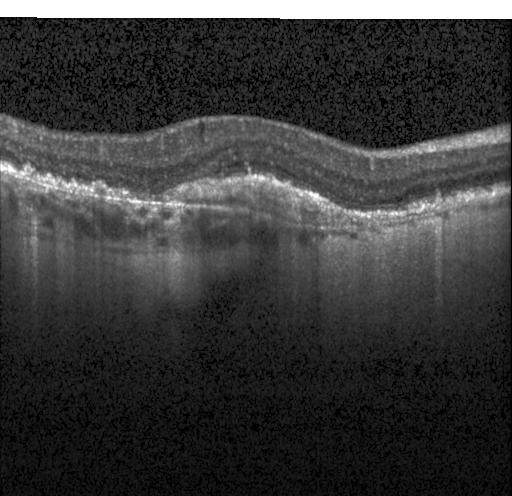

Choroidal neovascularization (CNV).